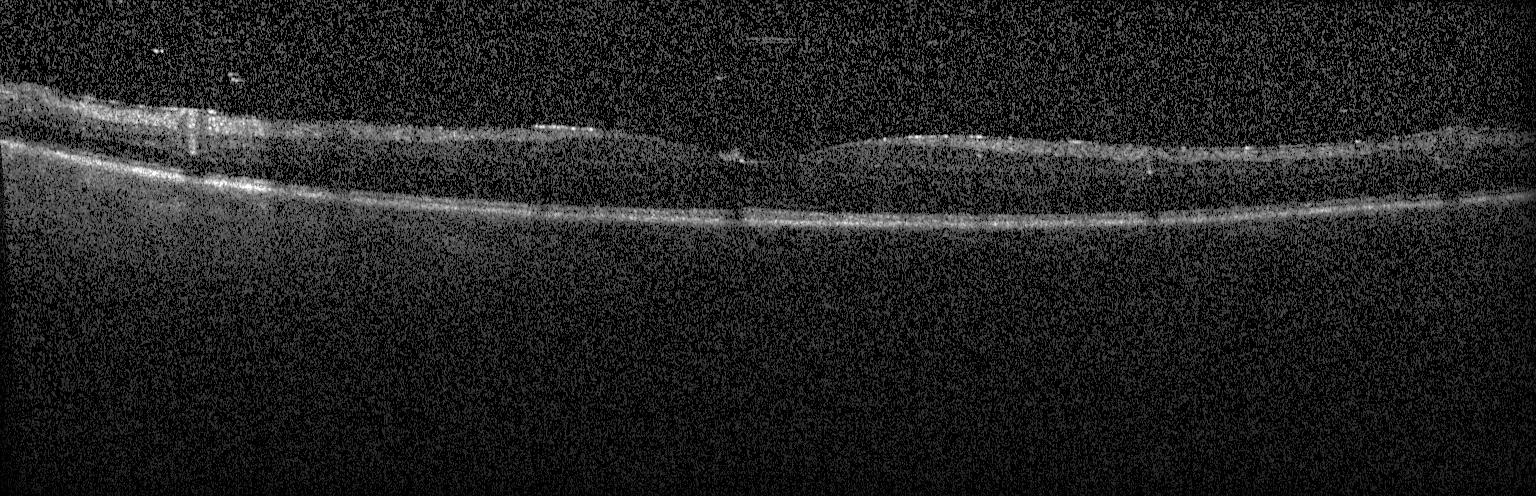
SD-OCT; optical coherence tomography B-scan.
Macular OCT: neither choroidal neovascularization, diabetic macular edema, nor drusen.